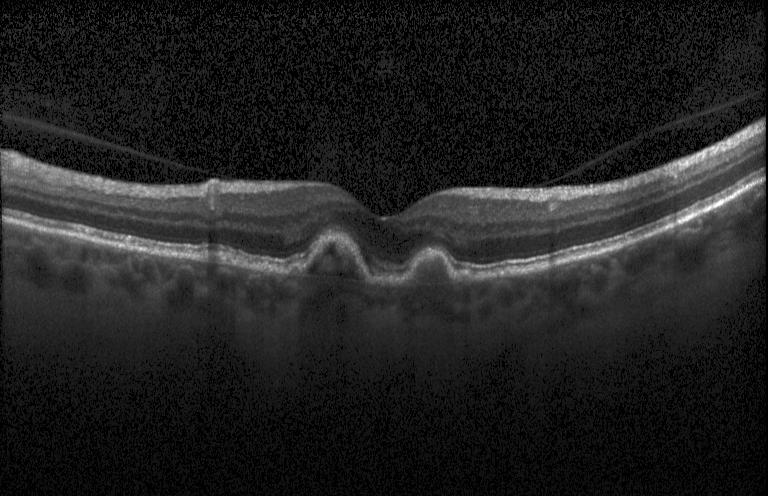

Spectral-domain OCT B-scan: drusen.